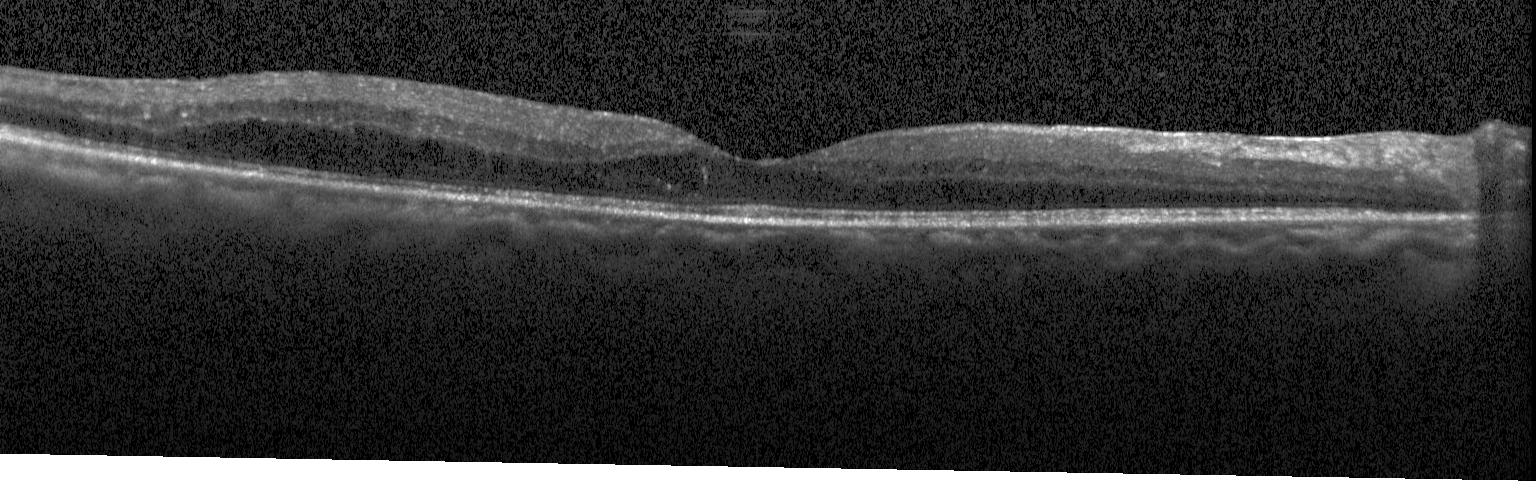

Retinal OCT cross-section showing DME.